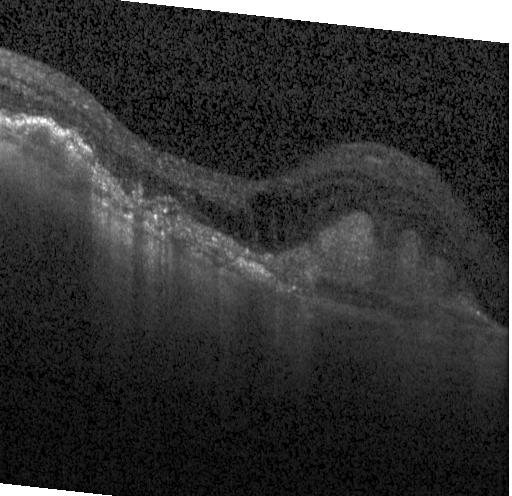

SD-OCT, OCT B-scan, centered on the fovea
This B-scan demonstrates choroidal neovascularization.